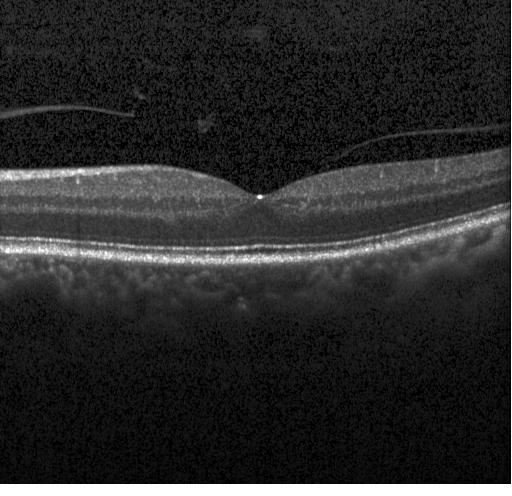

Diagnosis: no choroidal neovascularization, no diabetic macular edema, and no drusen.